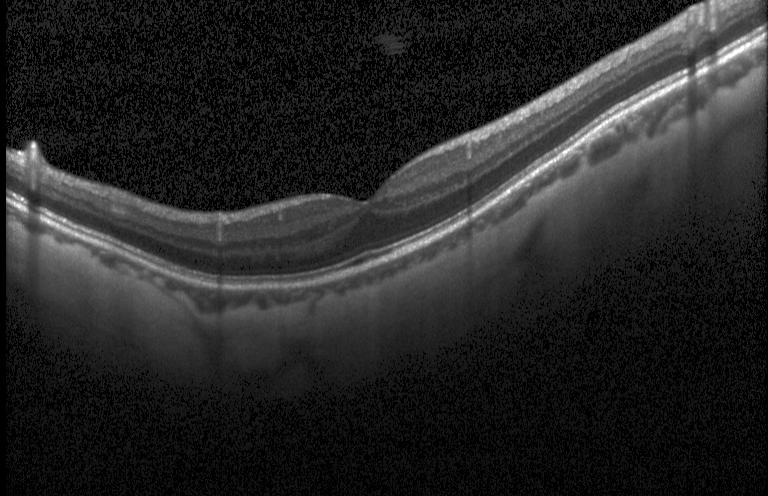

Spectral-domain OCT B-scan: neither choroidal neovascularization, diabetic macular edema, nor drusen.